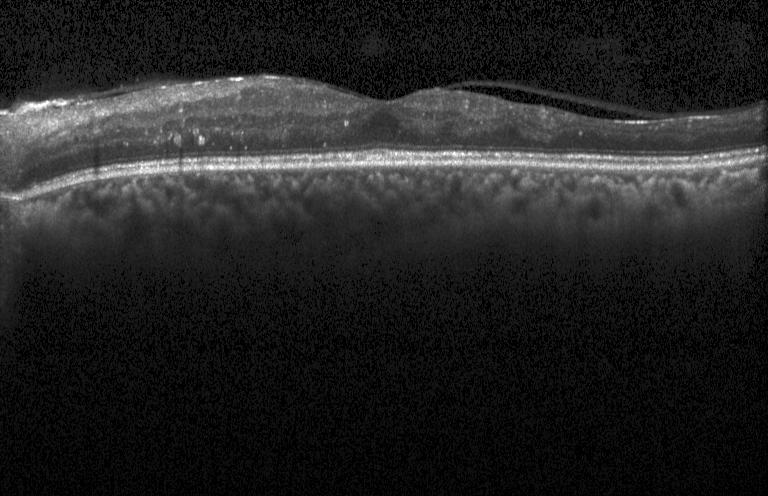 OCT finding: diabetic macular edema.